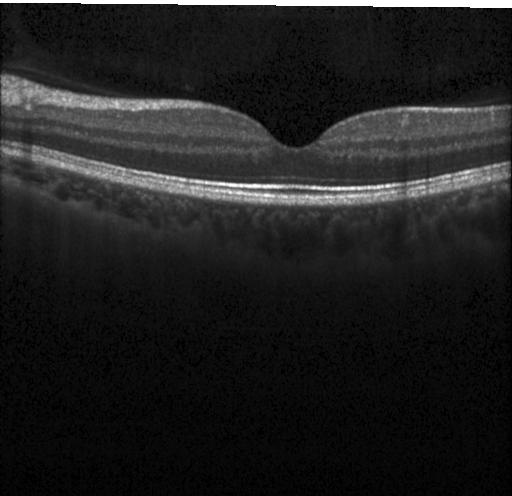 OCT line scan. Through the macula. Heidelberg Spectralis OCT system. SD-OCT
The scan shows no evidence of choroidal neovascularization, diabetic macular edema, or drusen.